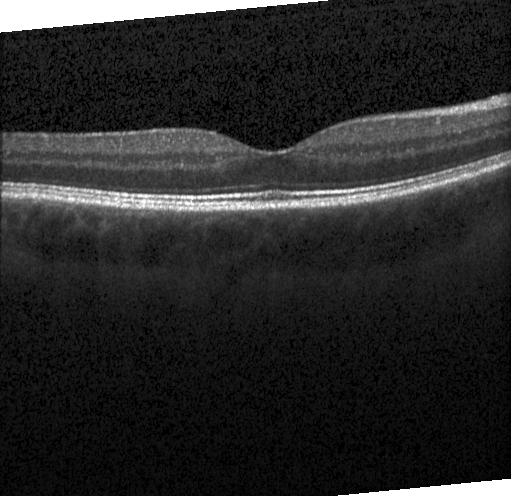

The scan shows no choroidal neovascularization, no diabetic macular edema, and no drusen.